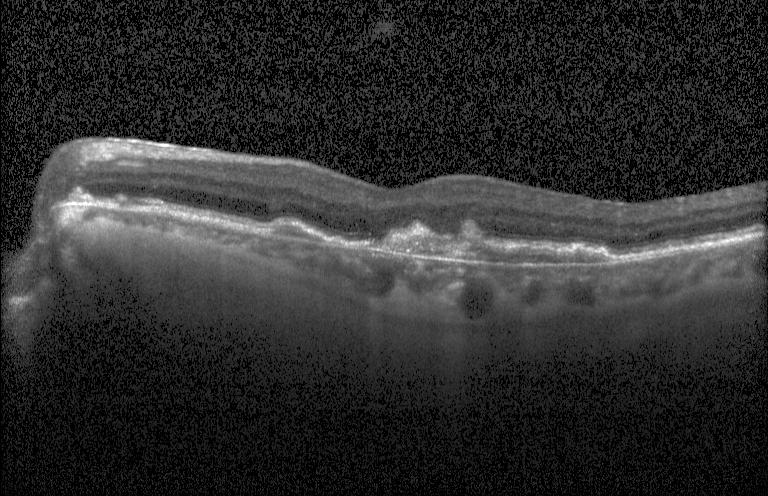
Optical coherence tomography scan. Spectral-domain optical coherence tomography.
Diagnosis: choroidal neovascularization (CNV).